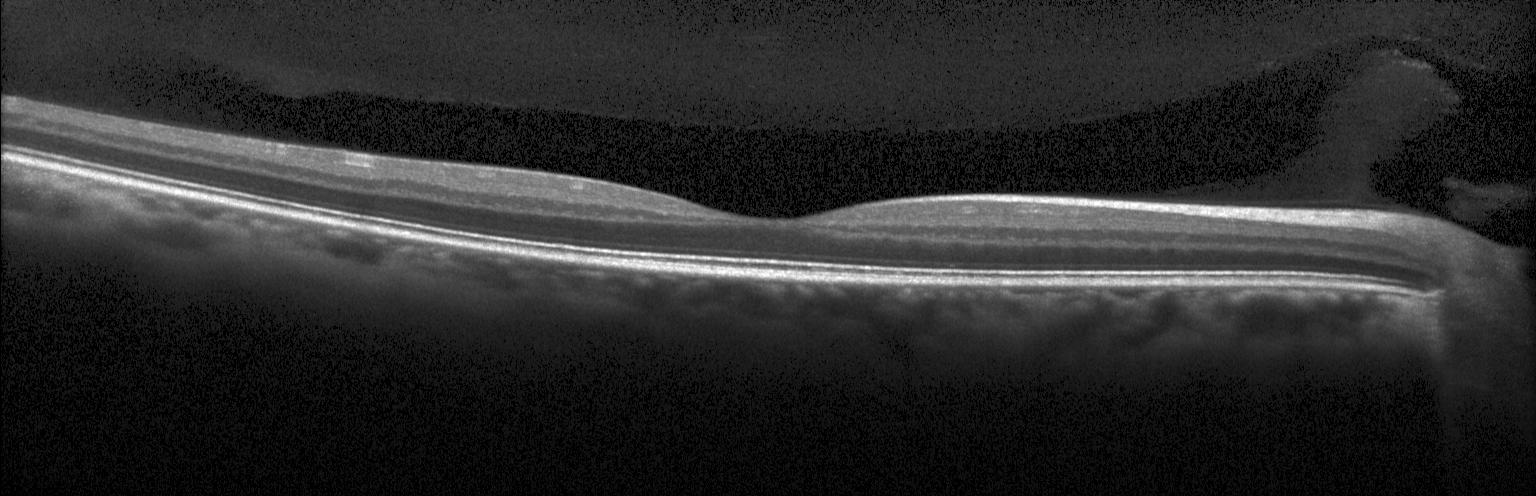
Dx: no CNV, DME, or drusen.